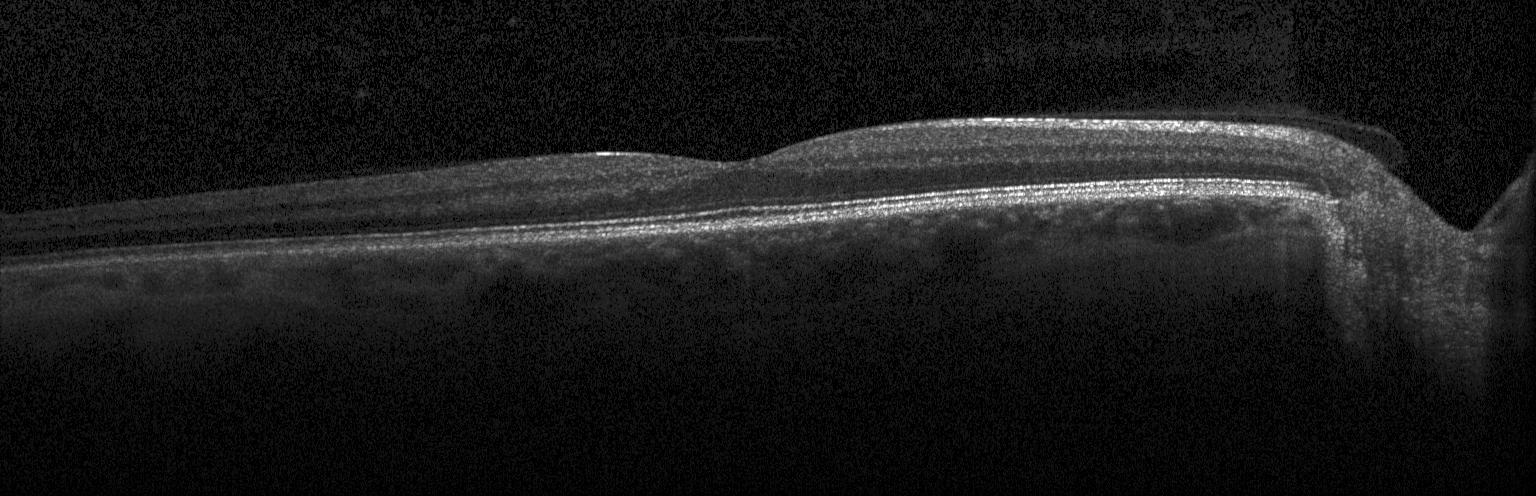
Impression: neither choroidal neovascularization, diabetic macular edema, nor drusen.